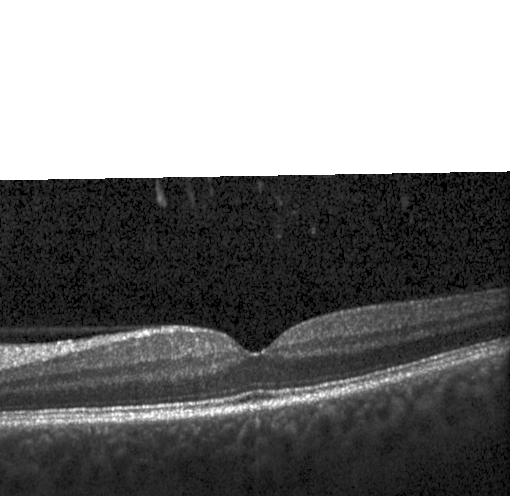 Optical coherence tomography B-scan; macular scan; Heidelberg Spectralis OCT system — Diagnosis: no choroidal neovascularization, diabetic macular edema, or drusen.